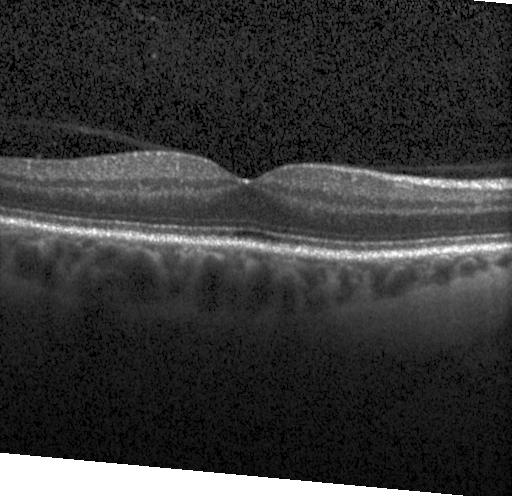

No evidence of CNV, DME, or drusen.